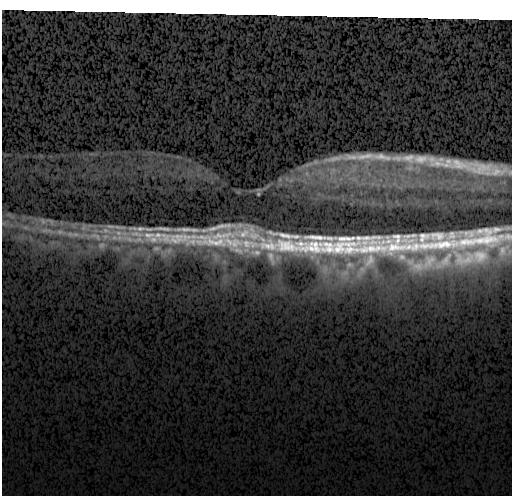
Spectral-domain OCT; instrument: Heidelberg Spectralis; fovea-centered; retinal OCT cross-section
Macular OCT: no choroidal neovascularization, no diabetic macular edema, and no drusen.